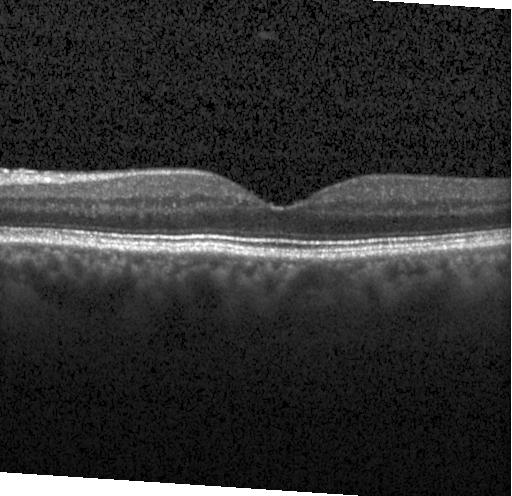

Acquired on a Heidelberg Spectralis · spectral-domain OCT · OCT line scan · fovea-centered — Macular OCT: no choroidal neovascularization, diabetic macular edema, or drusen.